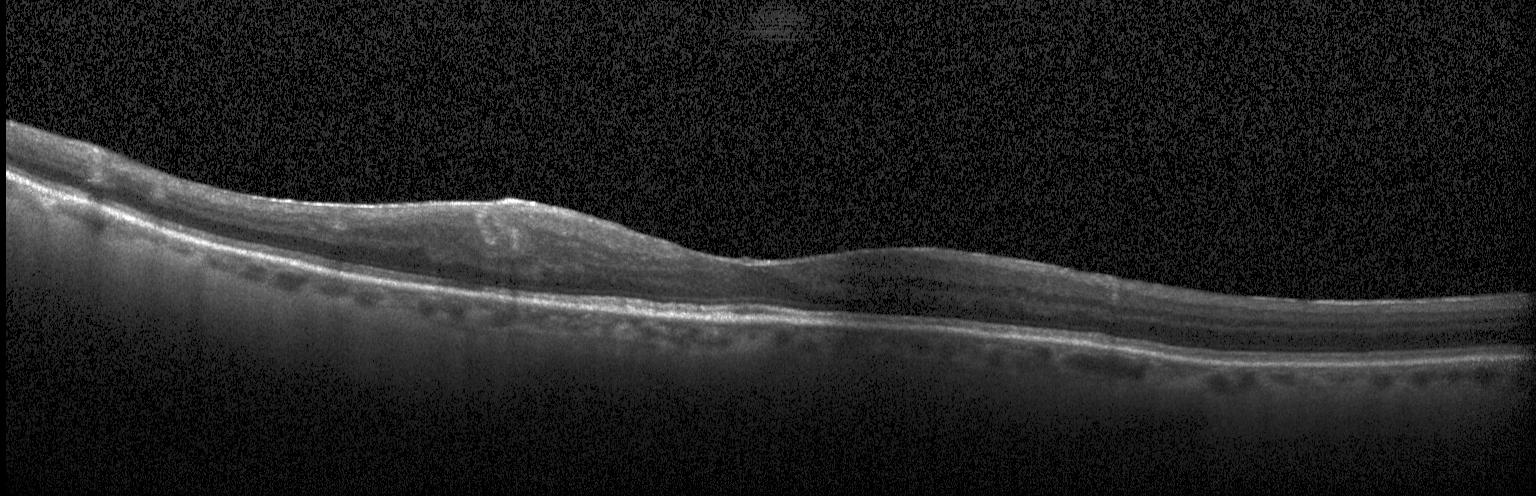

OCT finding: no CNV, no DME, and no drusen.